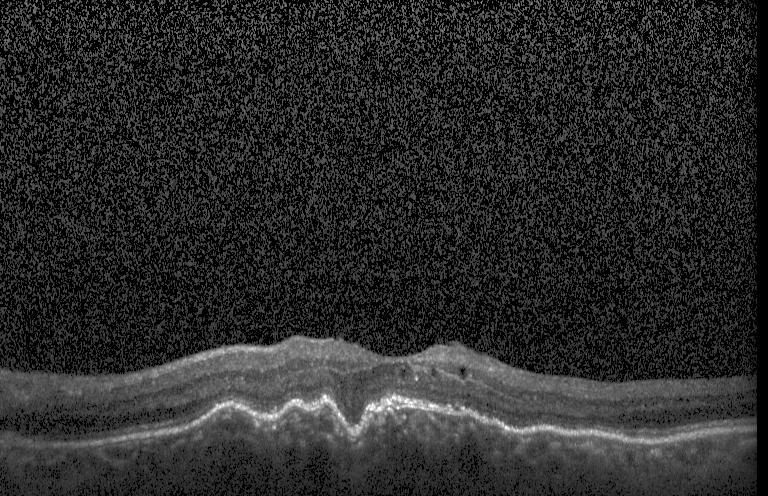

Optical coherence tomography scan; acquired on a Heidelberg Spectralis. Macular OCT: choroidal neovascularization.